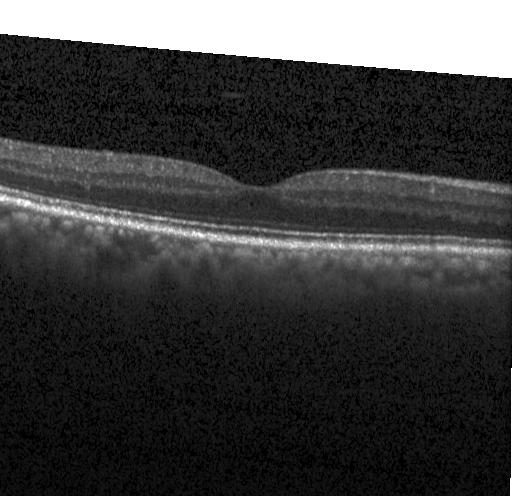
Spectral-domain OCT · OCT line scan. Macular OCT: no evidence of choroidal neovascularization, diabetic macular edema, or drusen.